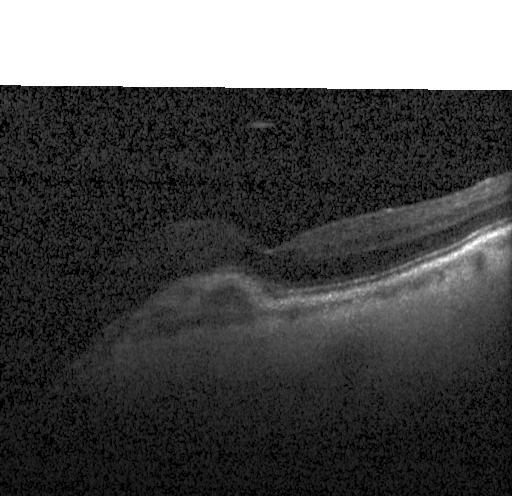
Through the macula · instrument: Heidelberg Spectralis · retinal OCT cross-section · spectral-domain OCT.
Assessment: CNV.